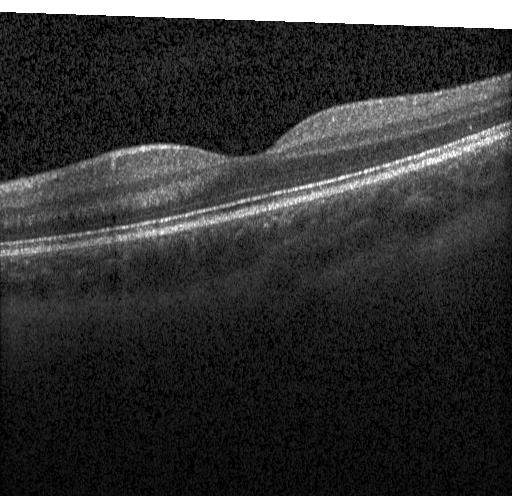
SD-OCT · OCT B-scan
This B-scan demonstrates no CNV, no DME, and no drusen.